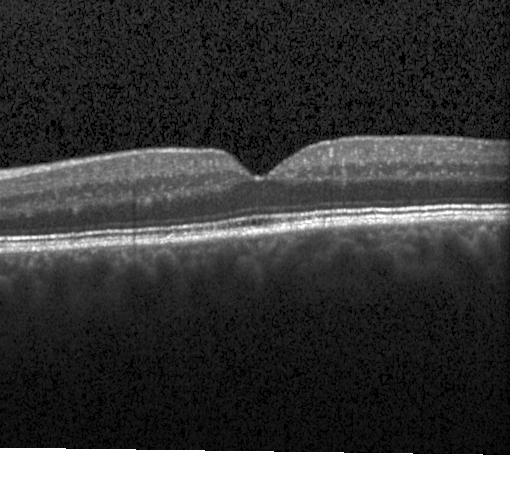
Finding: neither choroidal neovascularization, diabetic macular edema, nor drusen.